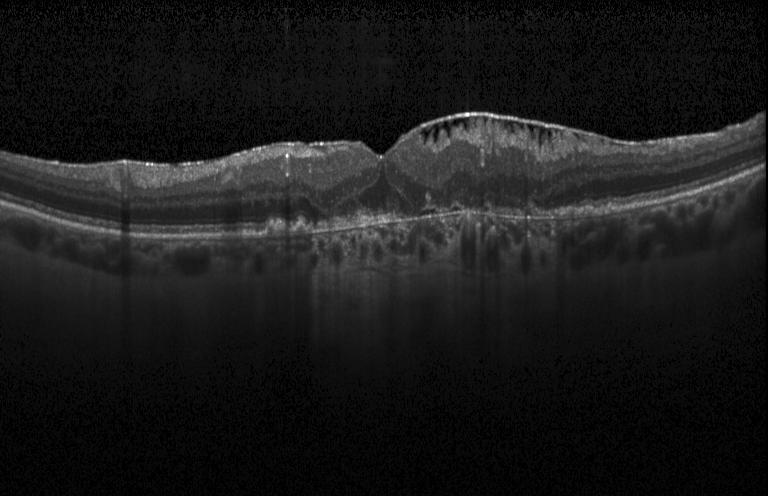 Centered on the fovea · OCT line scan — OCT finding: a choroidal neovascular membrane.